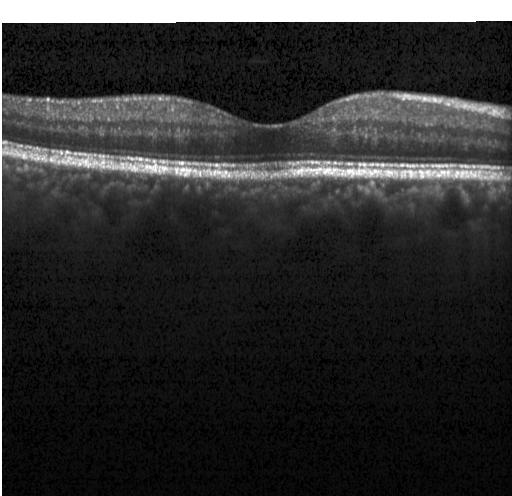 Horizontal scan through the fovea, OCT line scan.
The scan shows no CNV, no DME, and no drusen.